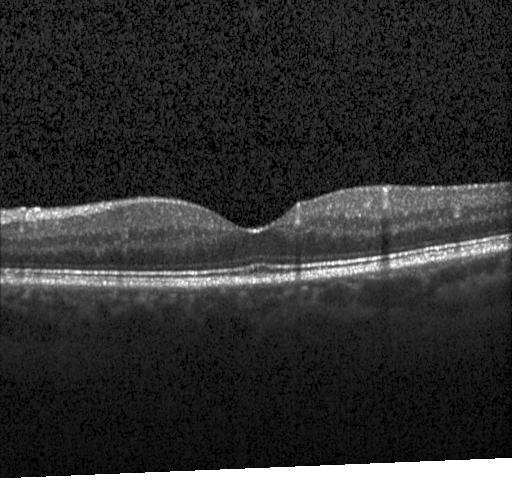
Assessment: neither choroidal neovascularization, diabetic macular edema, nor drusen.